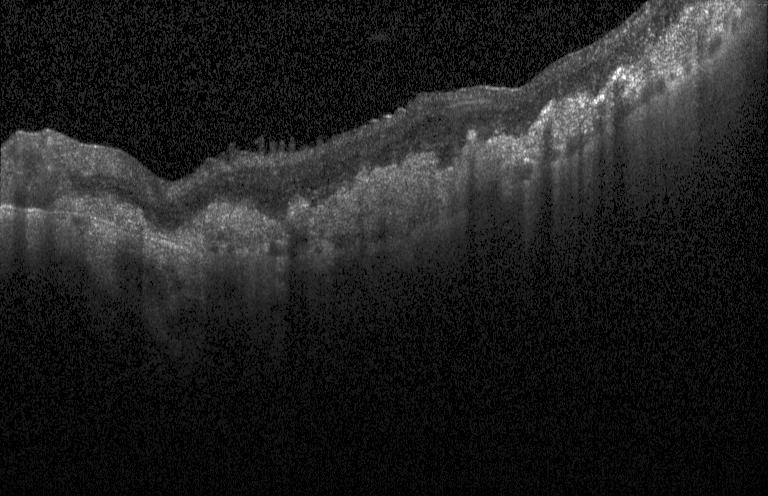
Heidelberg Spectralis OCT system. Retinal OCT cross-section. Spectral-domain OCT. Fovea-centered. Diagnosis: a choroidal neovascular membrane.